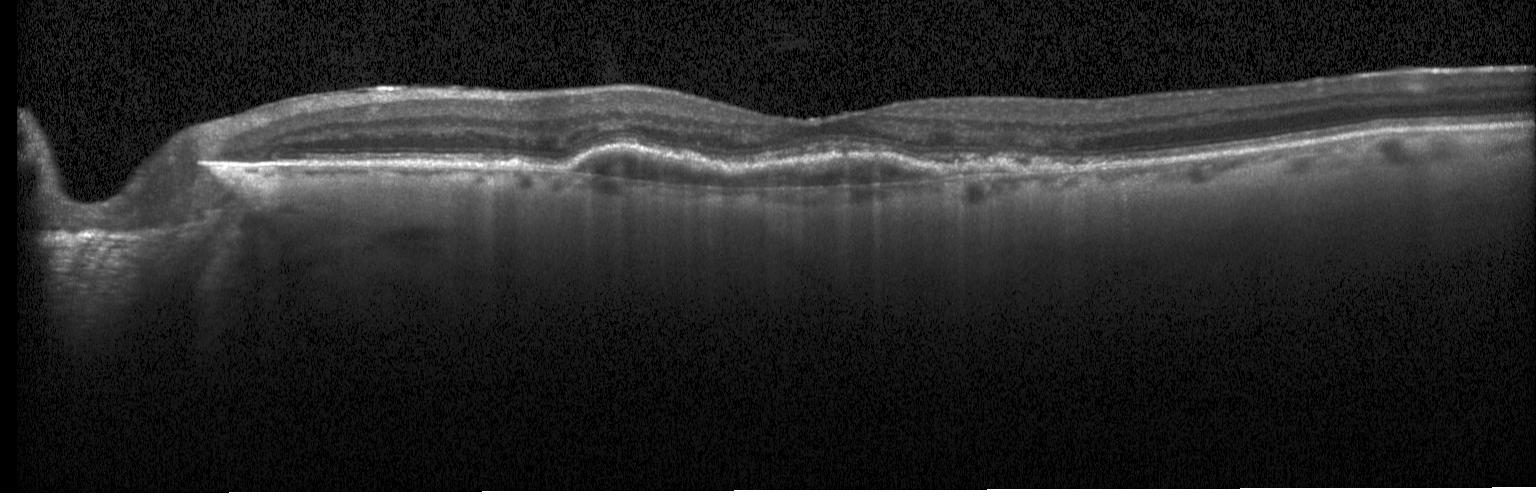
Retinal OCT cross-section.
Impression: a choroidal neovascular membrane.